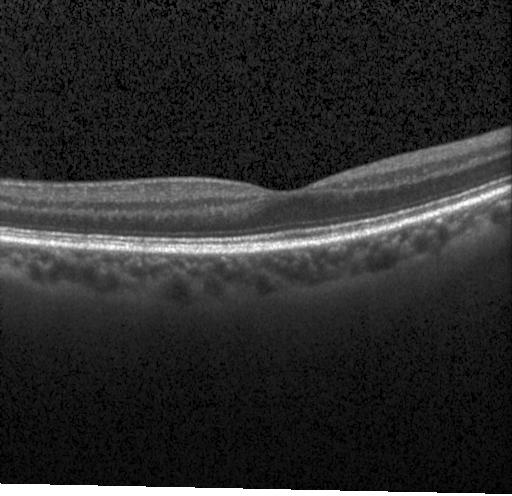
OCT scan showing no evidence of CNV, DME, or drusen.